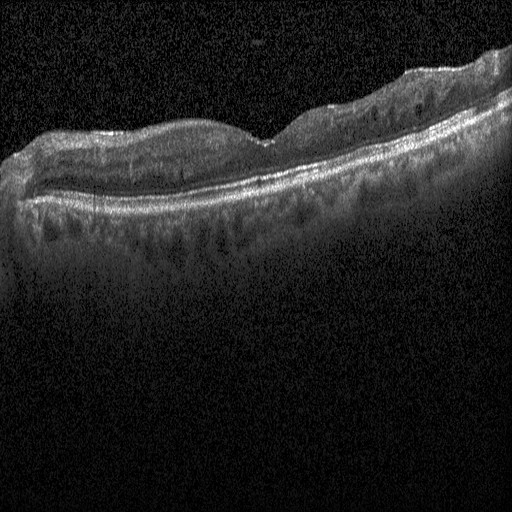
Acquired on a Heidelberg Spectralis, retinal OCT B-scan, horizontal scan through the fovea — Finding: diabetic macular edema (DME).